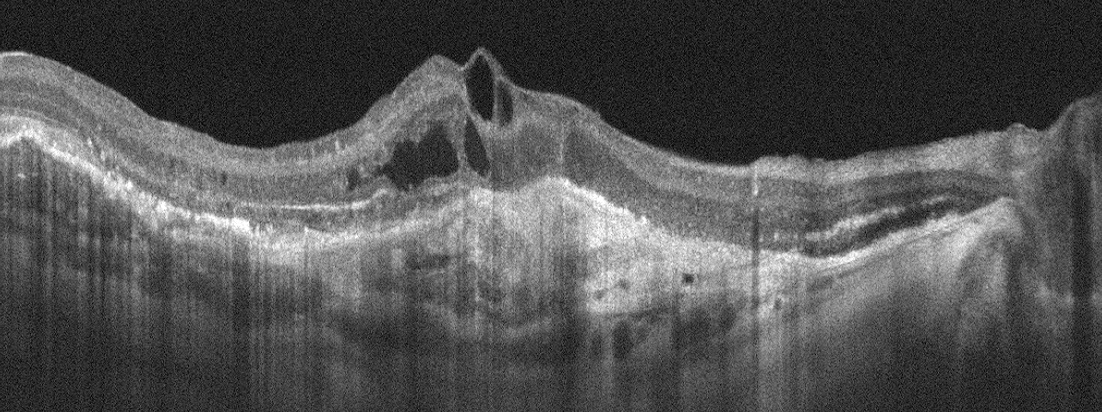

Macular OCT: age-related macular degeneration (AMD).